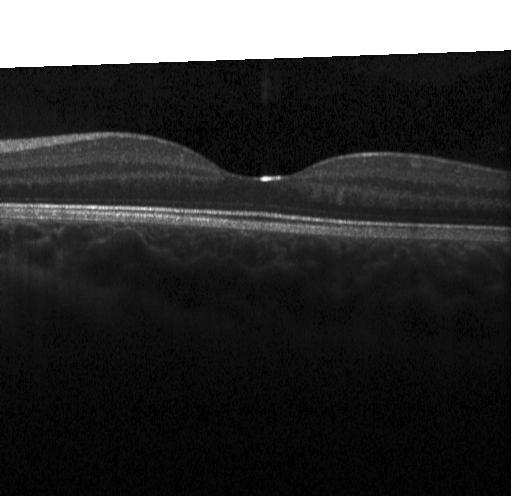 Macular OCT demonstrating no choroidal neovascularization, diabetic macular edema, or drusen.